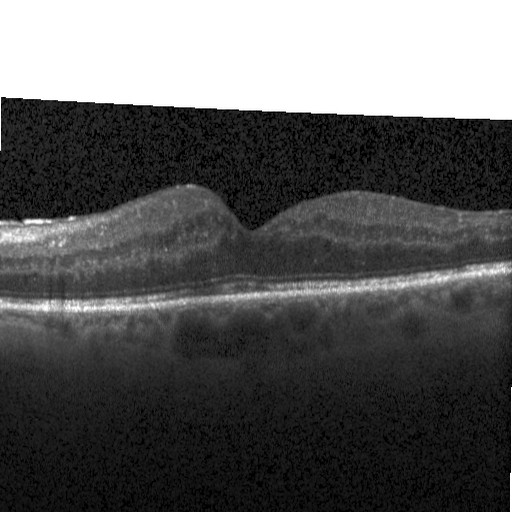

Instrument: Heidelberg Spectralis, optical coherence tomography scan — Macular OCT: diabetic macular edema (DME).